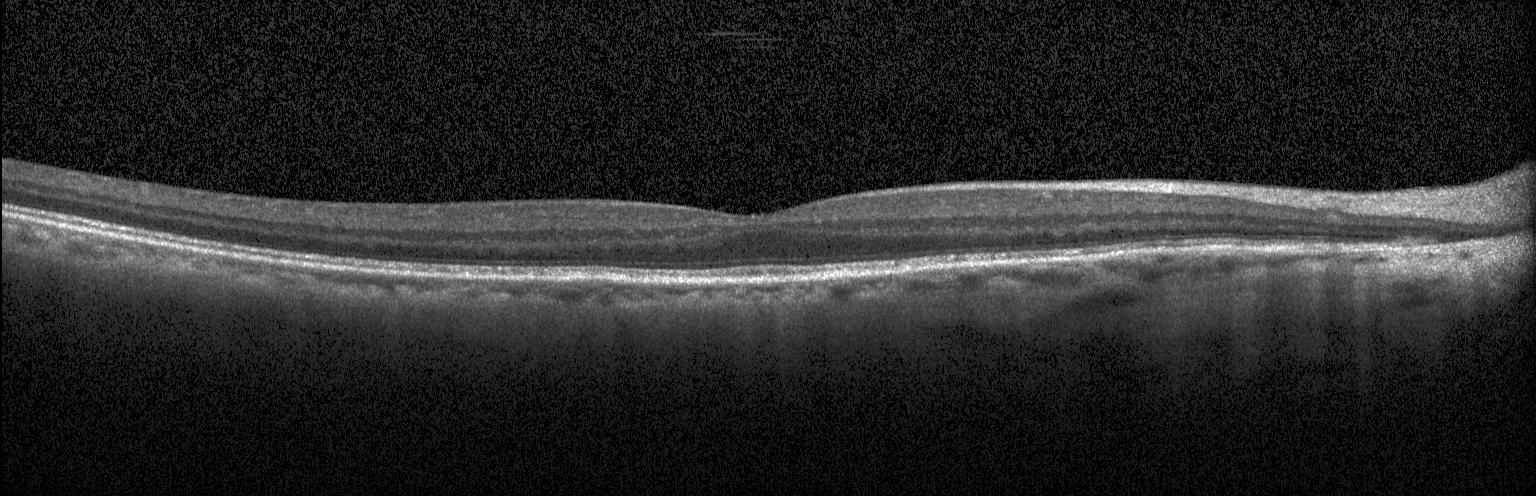 Through the macula; OCT B-scan; acquired on a Heidelberg Spectralis
This B-scan demonstrates no choroidal neovascularization, no diabetic macular edema, and no drusen.